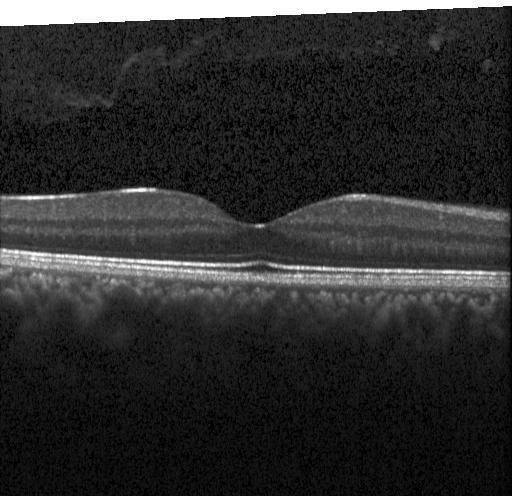
Finding: neither CNV, DME, nor drusen.